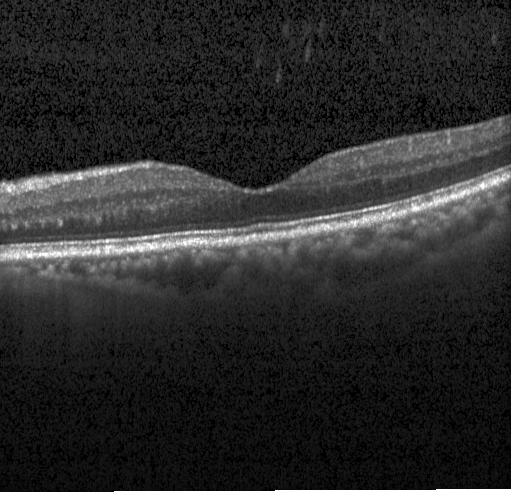
OCT scan showing neither CNV, DME, nor drusen.